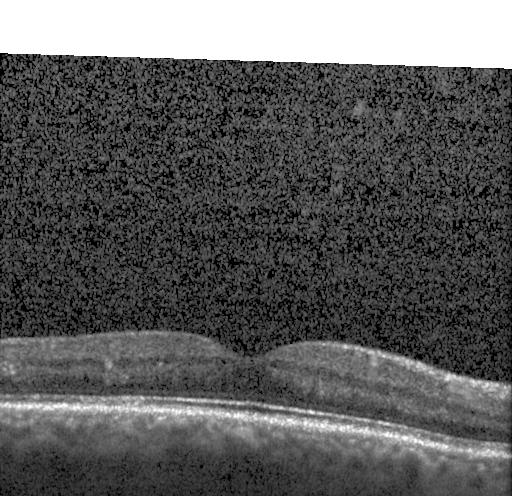

OCT B-scan
Macular OCT: neither CNV, DME, nor drusen.